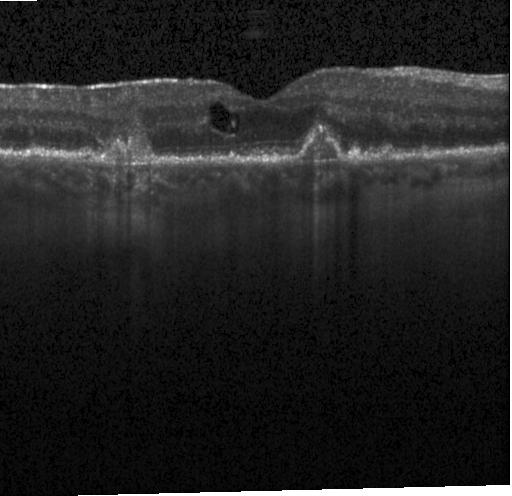 Heidelberg Spectralis OCT system · SD-OCT · retinal OCT B-scan · macular scan — CNV.